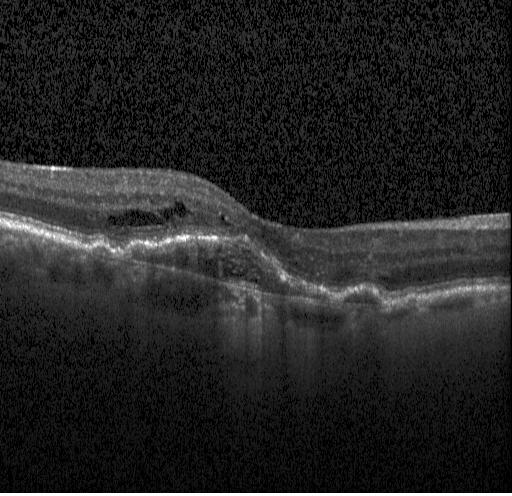

OCT B-scan, instrument: Heidelberg Spectralis — The scan shows a choroidal neovascular membrane.